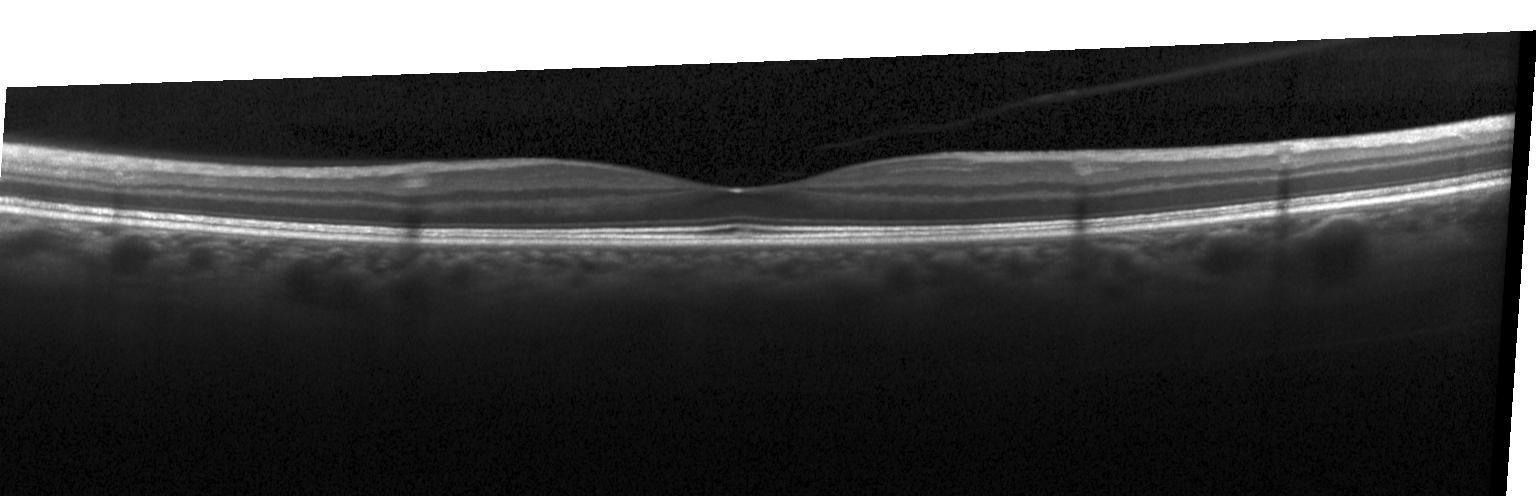

Fovea-centered. Spectral-domain OCT. Retinal OCT cross-section. Diagnosis: no evidence of CNV, DME, or drusen.